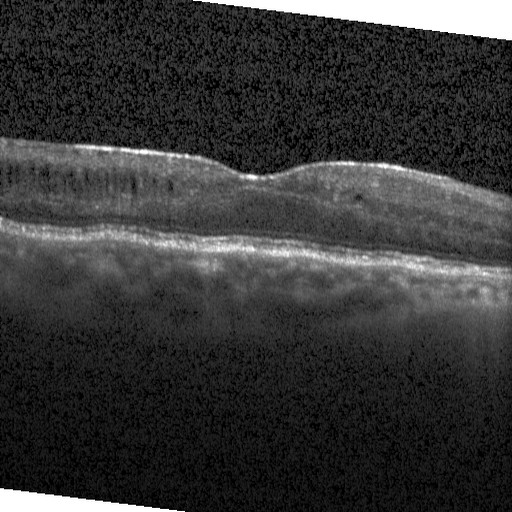 Optical coherence tomography B-scan. Diabetic macular edema.